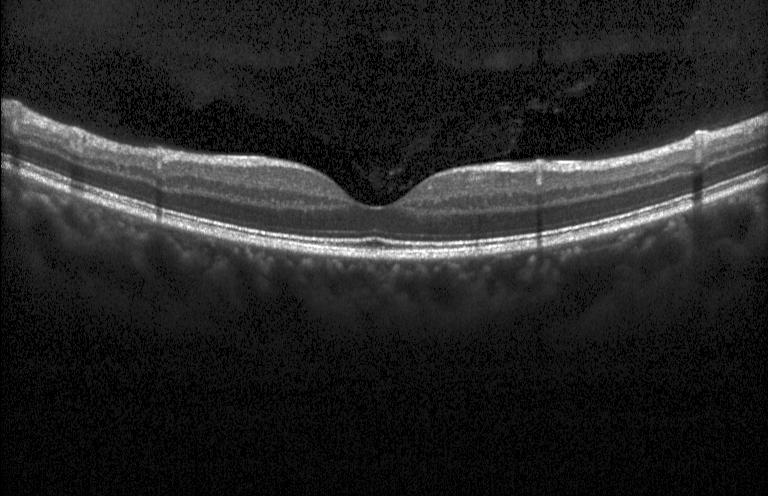 The scan shows no evidence of choroidal neovascularization, diabetic macular edema, or drusen.